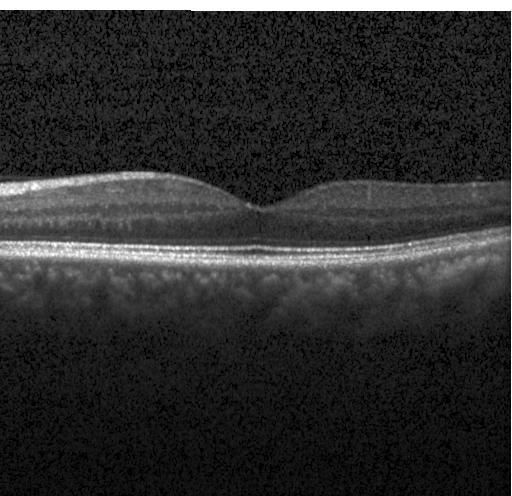

Diagnosis: no evidence of choroidal neovascularization, diabetic macular edema, or drusen.